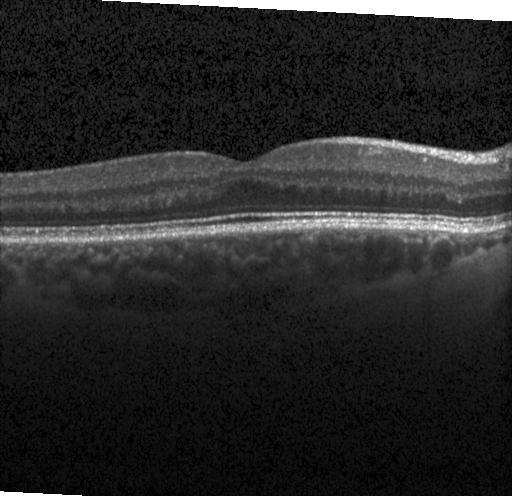
Impression: neither choroidal neovascularization, diabetic macular edema, nor drusen.